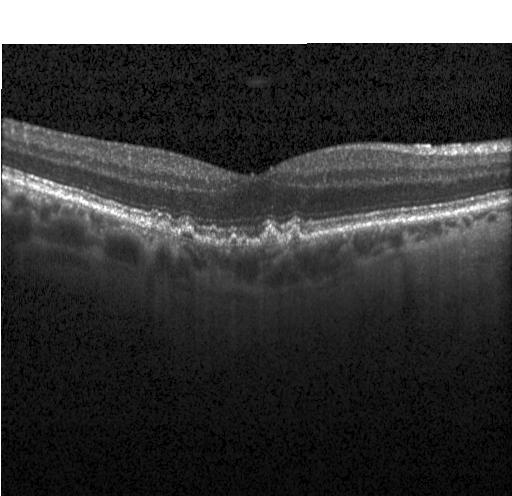 Fovea-centered; retinal OCT B-scan; SD-OCT; instrument: Heidelberg Spectralis.
Diagnosis: drusen.